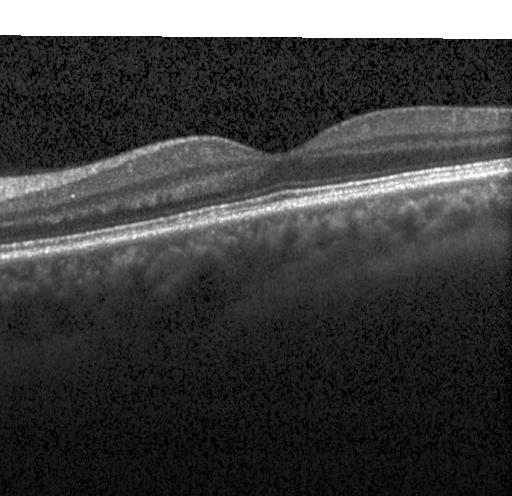

OCT line scan
Diagnosis: neither CNV, DME, nor drusen.